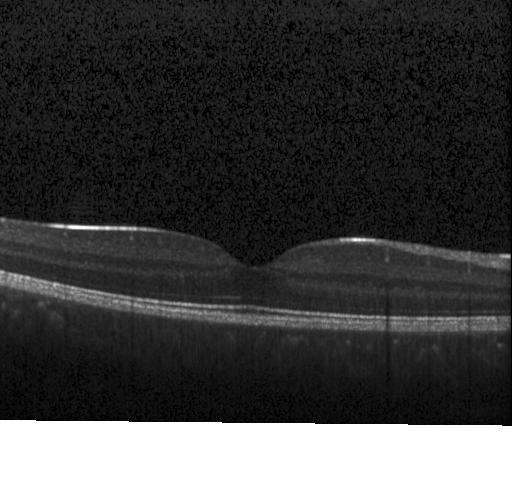
Retinal OCT cross-section · fovea-centered
OCT finding: no choroidal neovascularization, no diabetic macular edema, and no drusen.